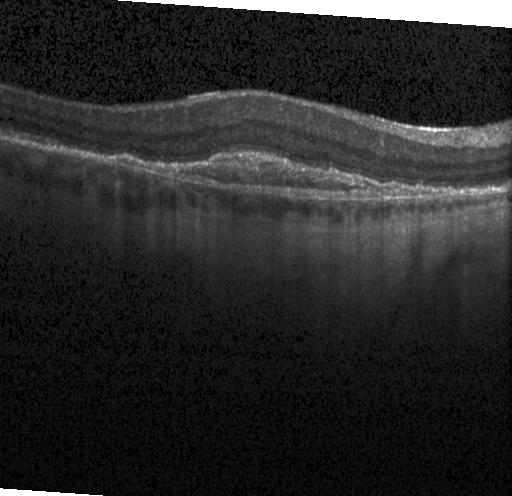

OCT B-scan · spectral-domain optical coherence tomography. Assessment: a choroidal neovascular membrane.